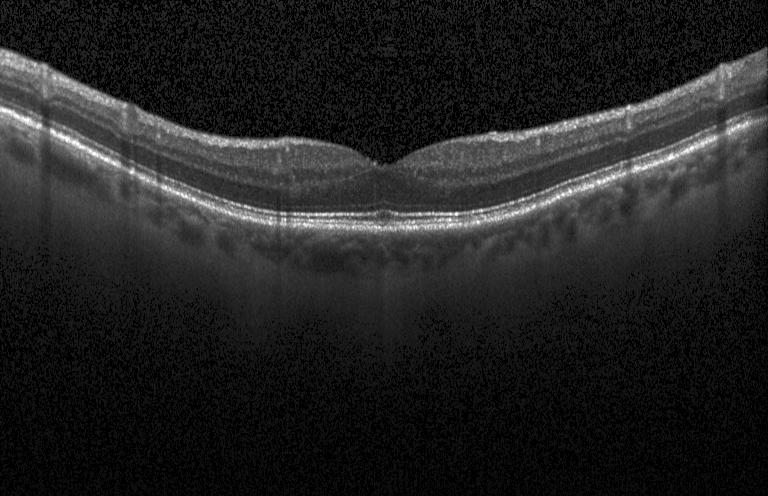
Spectral-domain OCT B-scan: no evidence of choroidal neovascularization, diabetic macular edema, or drusen.